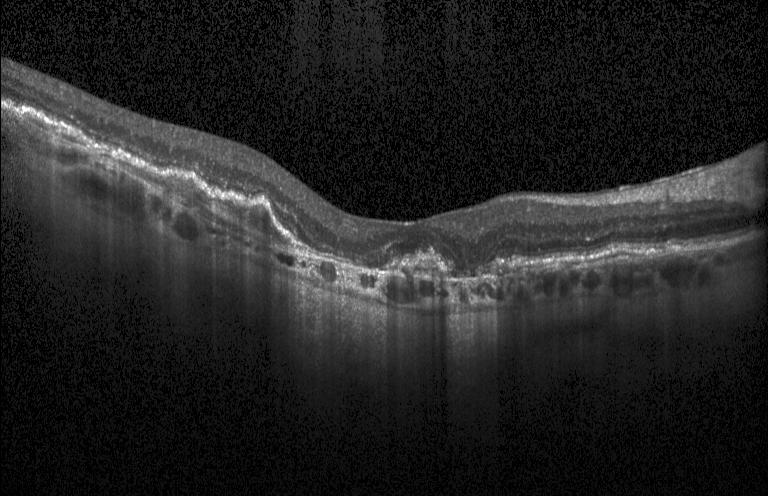 Spectral-domain OCT, OCT line scan, horizontal scan through the fovea, Heidelberg Spectralis OCT system
Impression: a choroidal neovascular membrane.